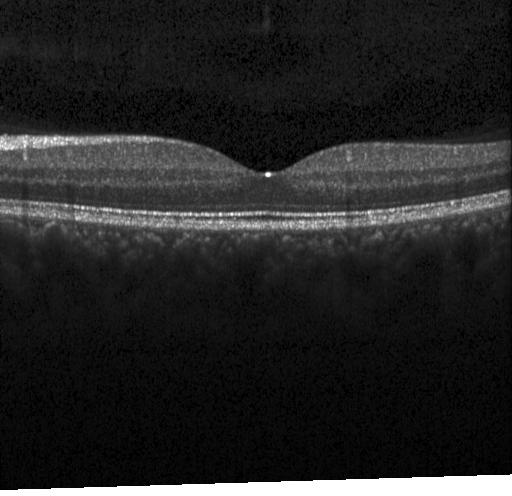

OCT line scan — The scan shows neither CNV, DME, nor drusen.